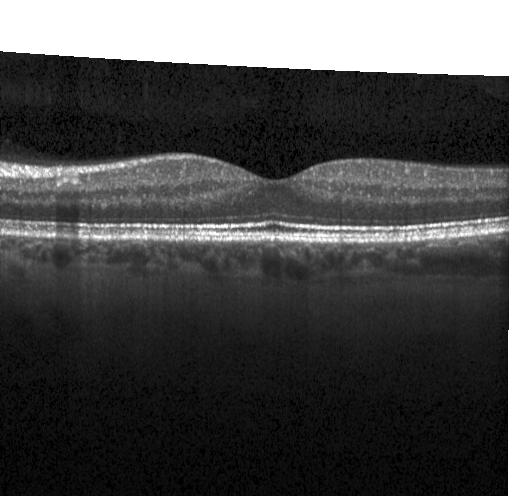
Impression: no evidence of choroidal neovascularization, diabetic macular edema, or drusen.